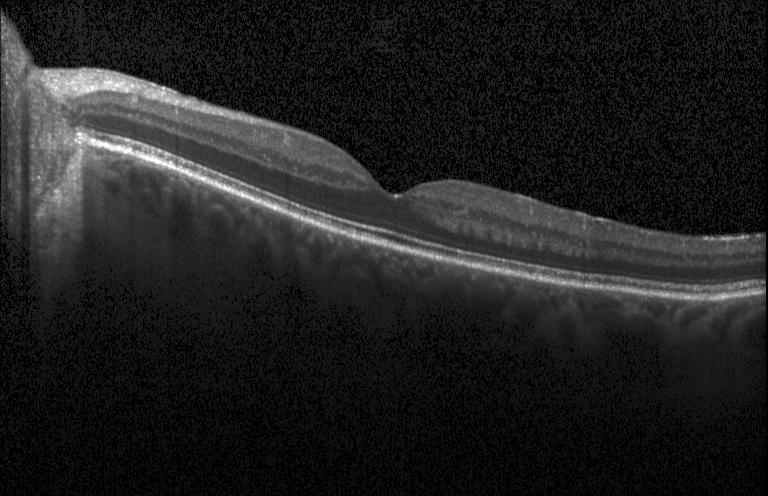 Centered on the fovea; OCT B-scan — The scan shows no choroidal neovascularization, no diabetic macular edema, and no drusen.